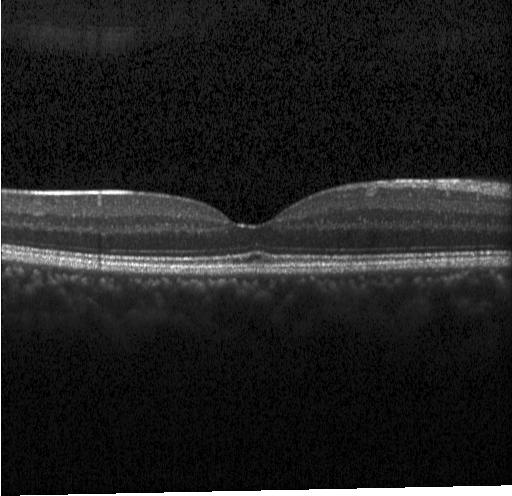

Impression: neither CNV, DME, nor drusen.